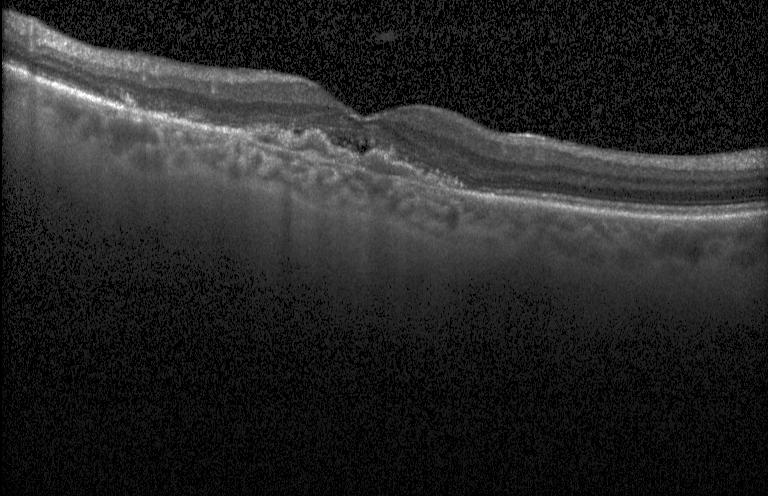 Through the macula. OCT line scan.
Finding: choroidal neovascularization (CNV).